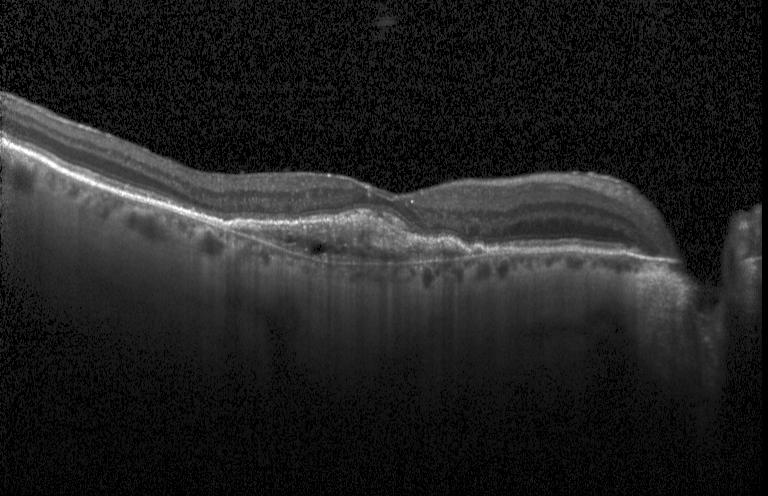

Optical coherence tomography scan
Diagnosis: choroidal neovascularization (CNV).